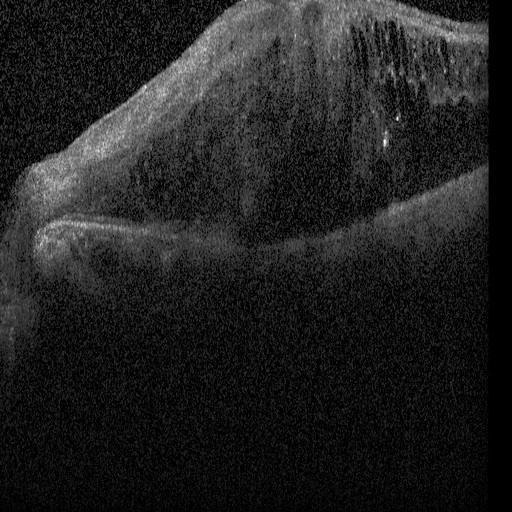
OCT B-scan
Macular OCT: DME.